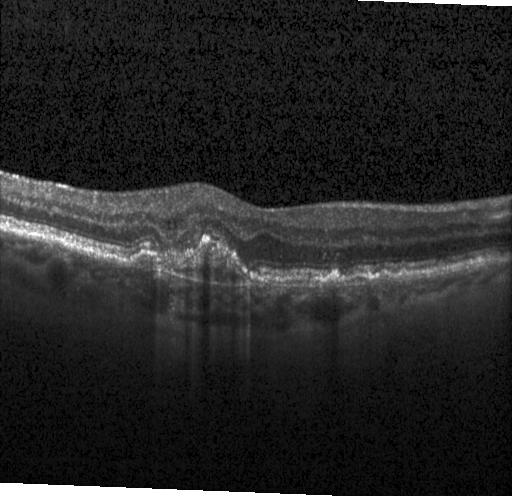
OCT scan showing CNV.